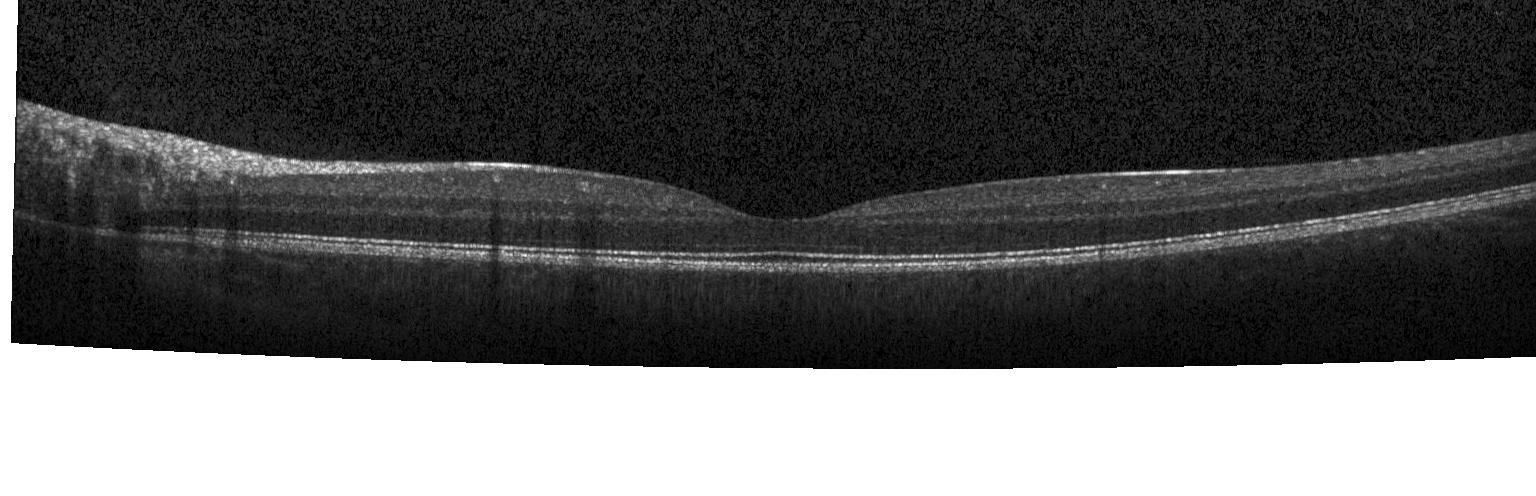
Impression: no evidence of choroidal neovascularization, diabetic macular edema, or drusen.